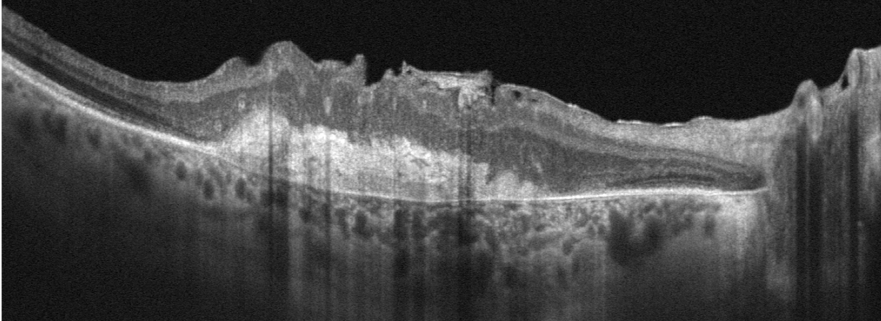 Diagnosis: age-related macular degeneration (AMD).